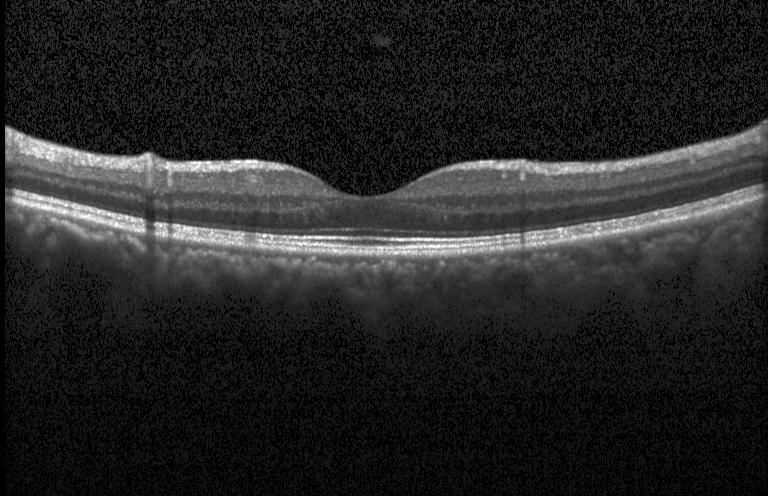 Assessment: no choroidal neovascularization, no diabetic macular edema, and no drusen.